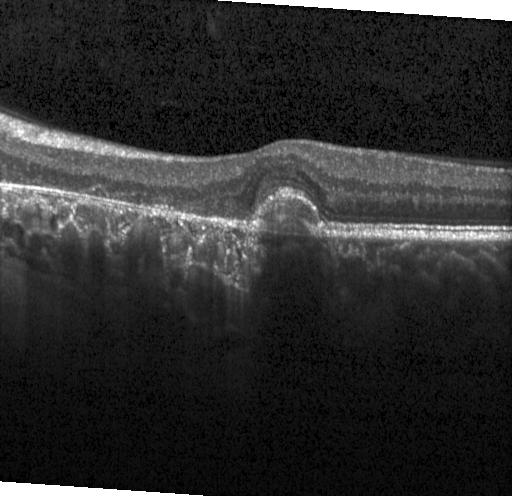 Optical coherence tomography scan.
Assessment: CNV.